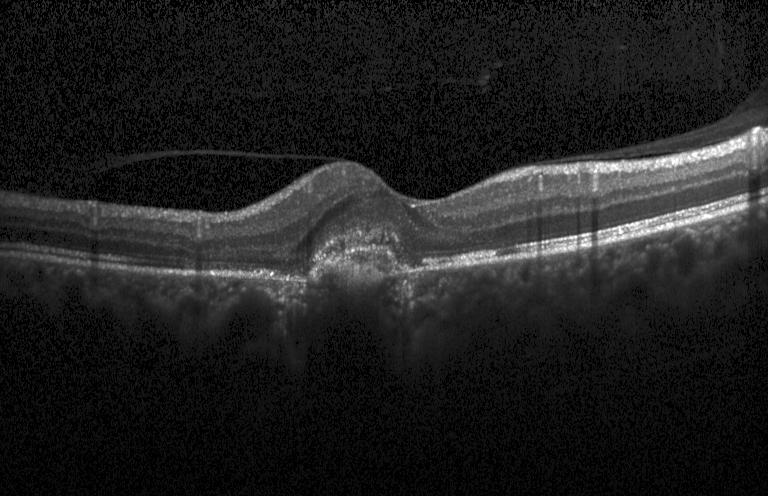
Retinal OCT cross-section. This B-scan demonstrates a choroidal neovascular membrane.